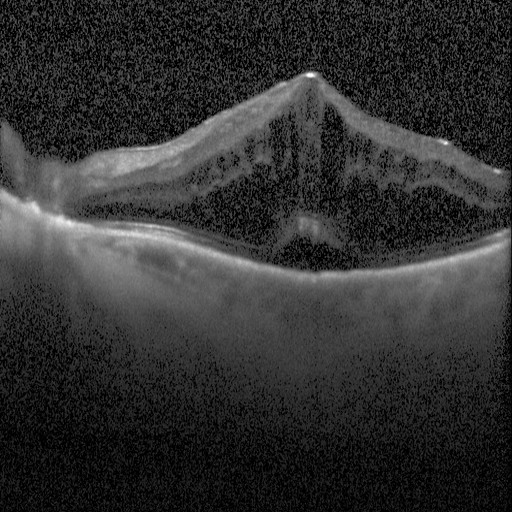

Optical coherence tomography B-scan, Heidelberg Spectralis
Finding: diabetic macular edema.